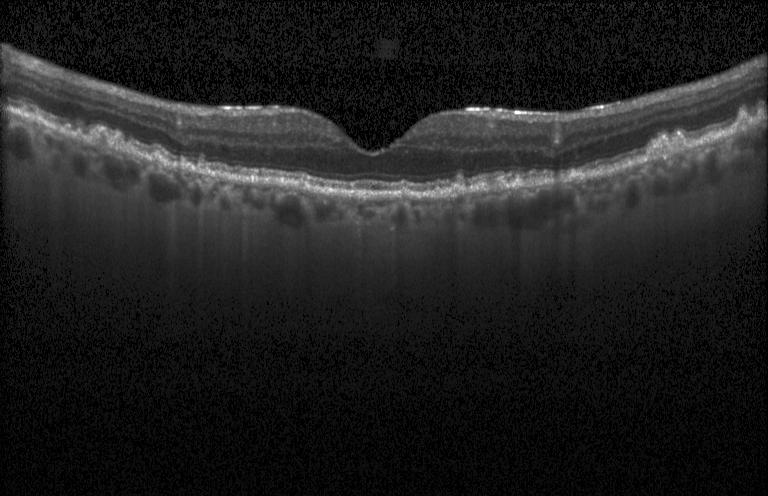 Macular OCT: multiple drusen.